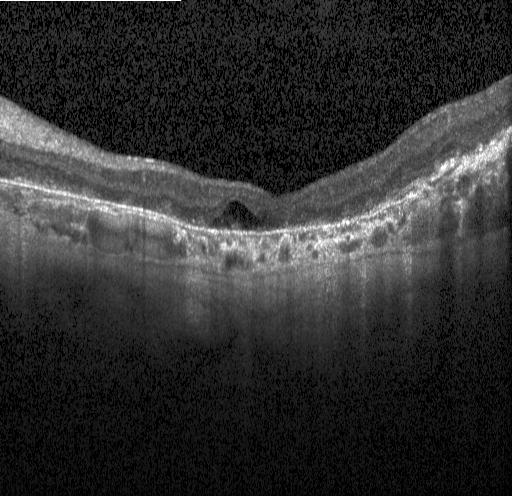
Optical coherence tomography scan
The scan shows choroidal neovascularization.